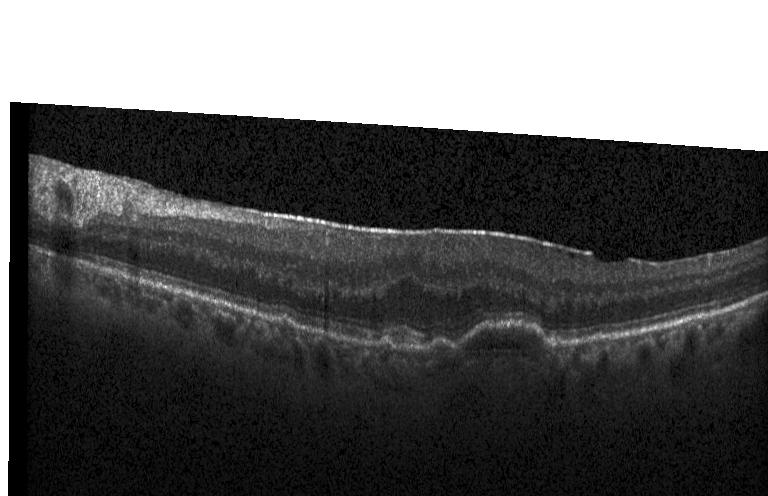

Centered on the fovea. Spectral-domain OCT. Retinal OCT B-scan.
This B-scan demonstrates choroidal neovascularization.